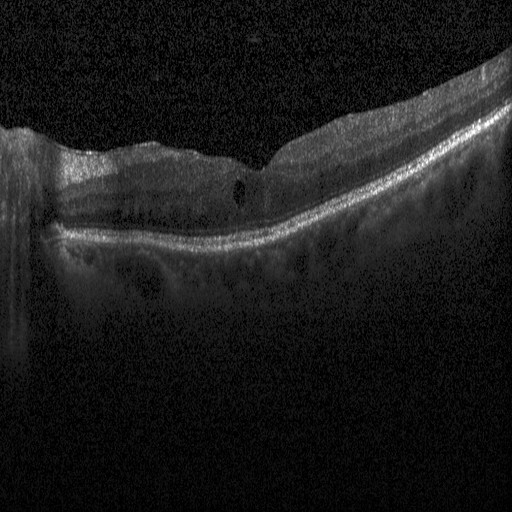

Acquired on a Heidelberg Spectralis, optical coherence tomography B-scan.
Diagnosis: DME.